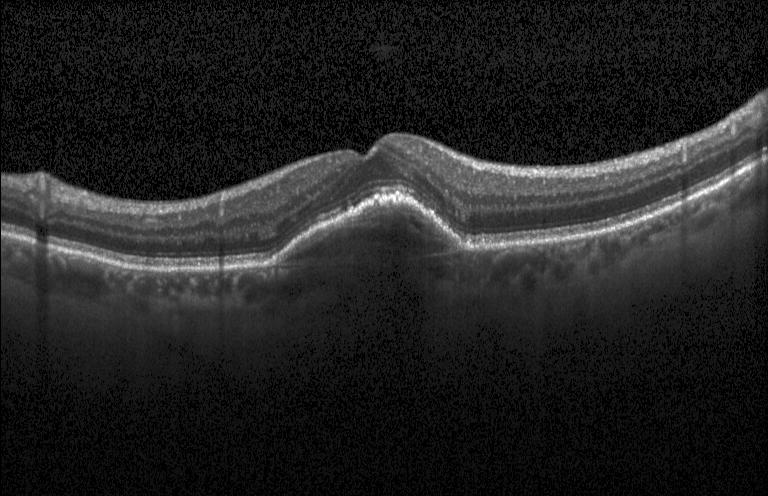
OCT B-scan; centered on the fovea; Heidelberg Spectralis
This B-scan demonstrates a choroidal neovascular membrane.